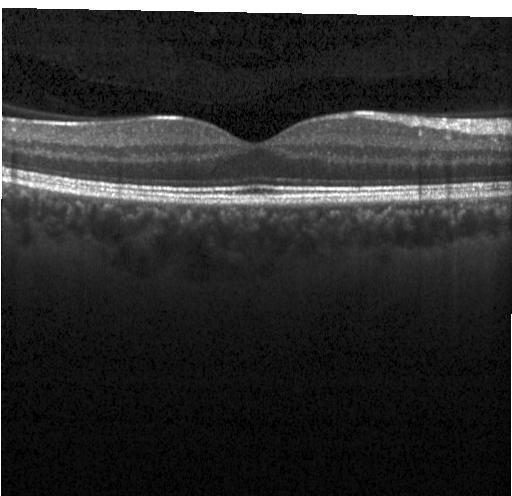

Retinal OCT cross-section showing no choroidal neovascularization, no diabetic macular edema, and no drusen.